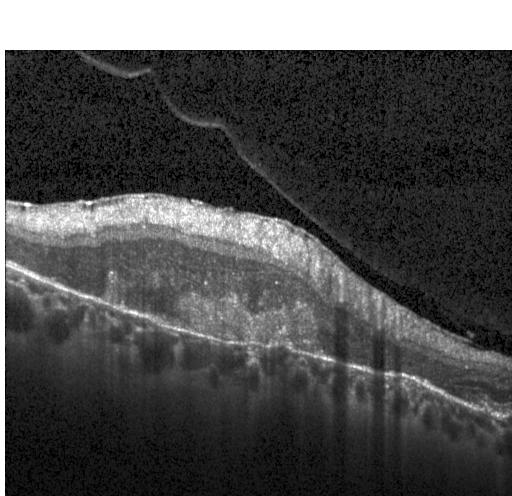 Spectral-domain OCT B-scan: a choroidal neovascular membrane.